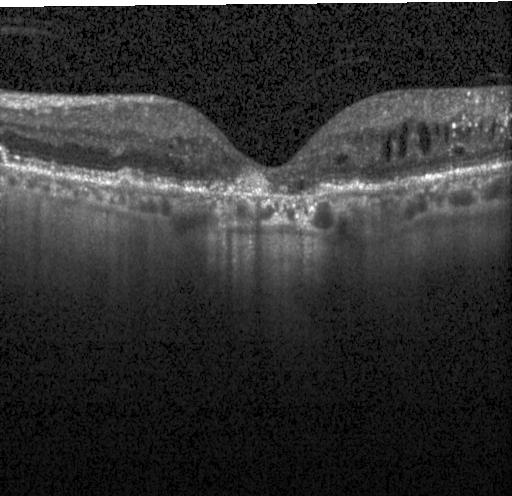 OCT finding: choroidal neovascularization (CNV).